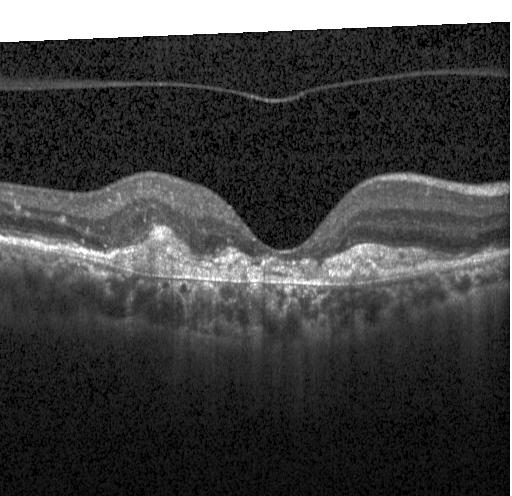 OCT B-scan. Instrument: Heidelberg Spectralis. Spectral-domain OCT. A choroidal neovascular membrane.